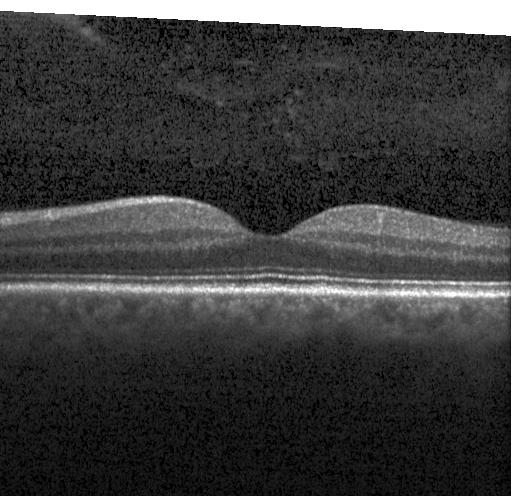

OCT B-scan showing neither CNV, DME, nor drusen.